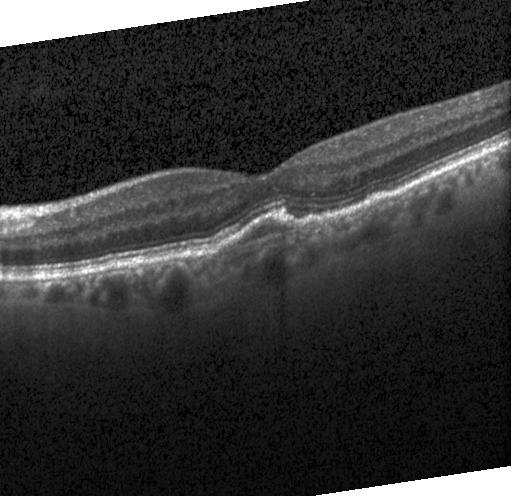

Instrument: Heidelberg Spectralis. Macular scan. Optical coherence tomography scan. Assessment: choroidal neovascularization (CNV).